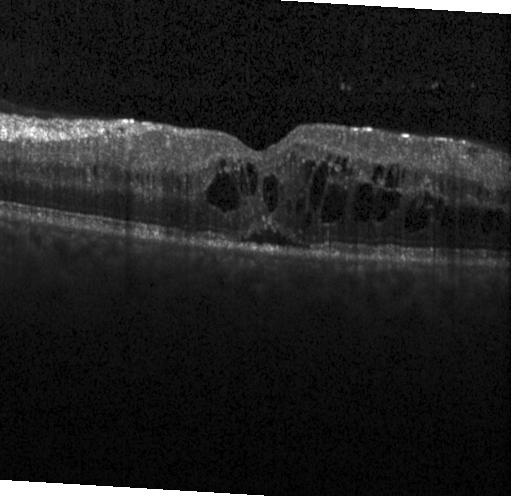

OCT line scan.
The scan shows DME.